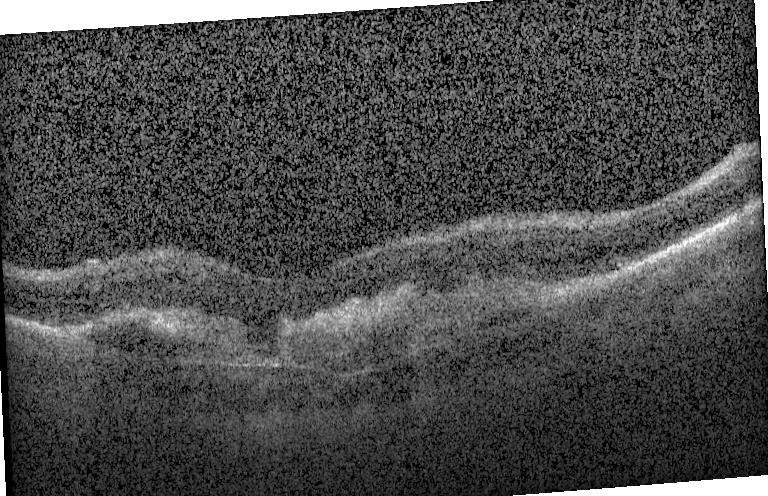
OCT line scan, spectral-domain OCT, Heidelberg Spectralis. Dx: CNV.